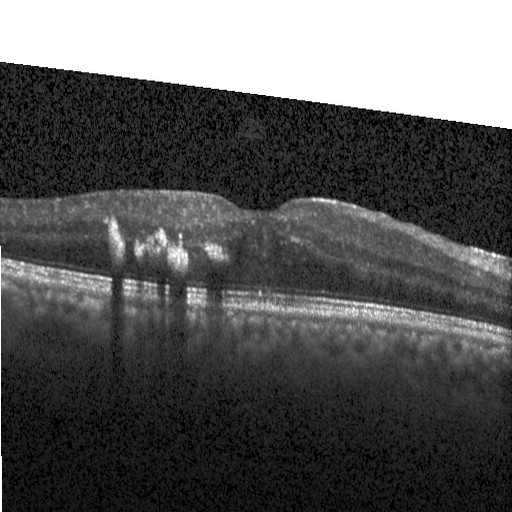 Retinal OCT B-scan. Through the macula.
Impression: diabetic macular edema (DME).